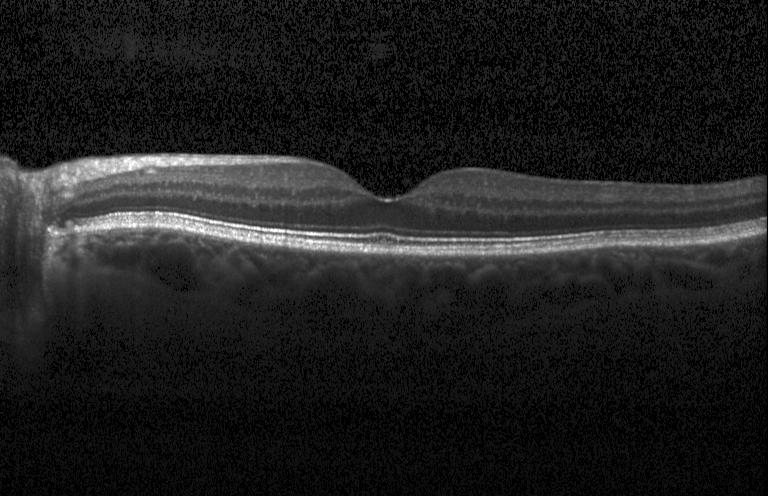

This B-scan demonstrates no choroidal neovascularization, no diabetic macular edema, and no drusen.